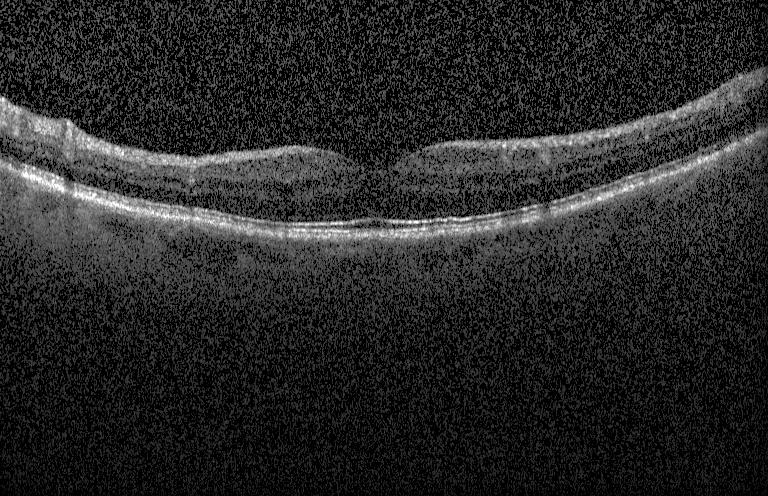
Impression: neither CNV, DME, nor drusen.